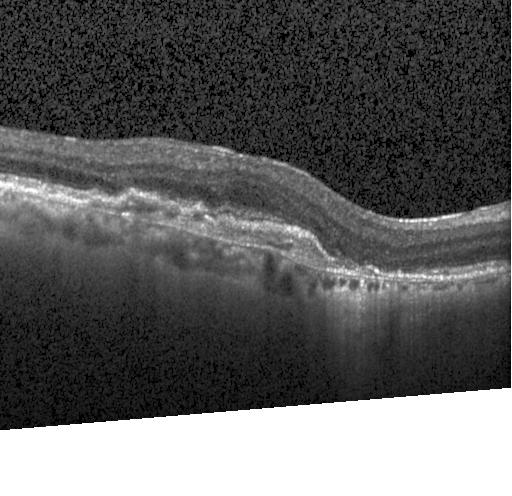

OCT line scan, centered on the fovea
Impression: CNV.